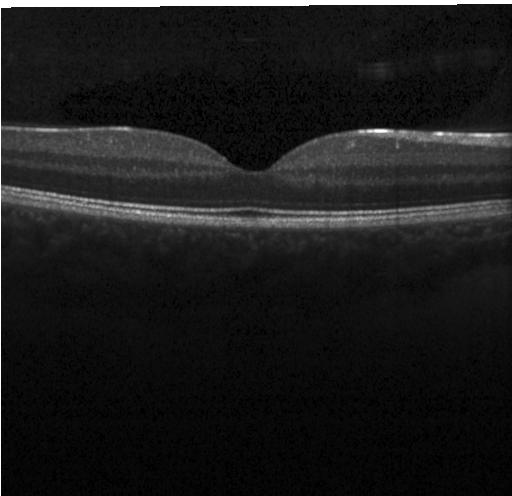
Through the macula · retinal OCT cross-section — The scan shows no evidence of choroidal neovascularization, diabetic macular edema, or drusen.